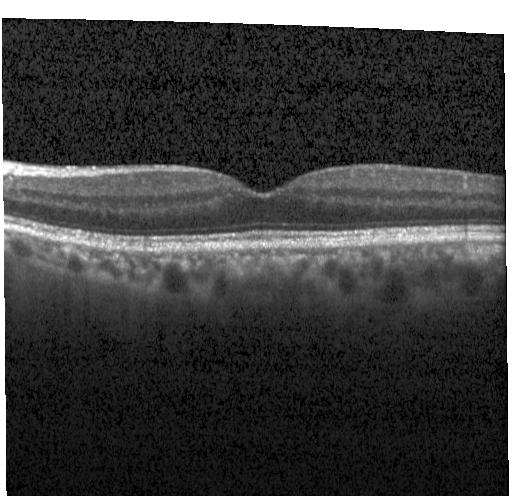
OCT B-scan. Heidelberg Spectralis. Finding: no choroidal neovascularization, diabetic macular edema, or drusen.